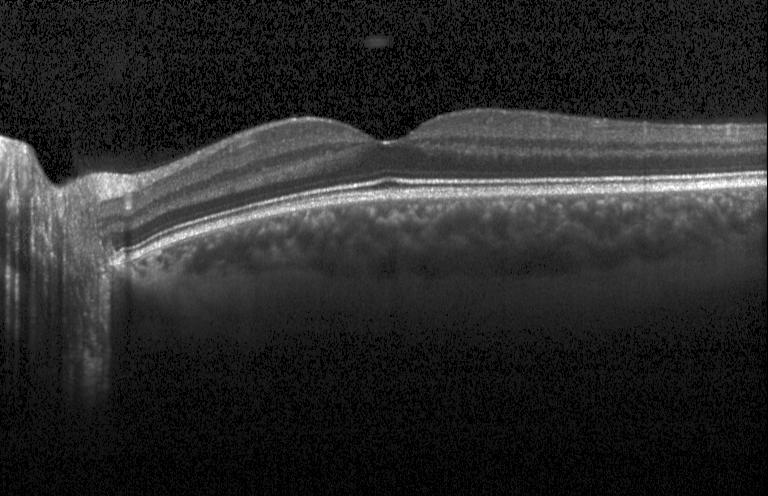
Instrument: Heidelberg Spectralis · macular scan · retinal OCT cross-section · spectral-domain optical coherence tomography — Diagnosis: neither CNV, DME, nor drusen.